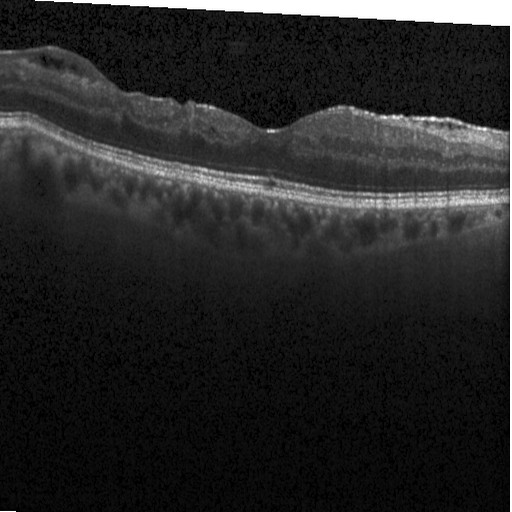
OCT finding: diabetic macular edema (DME).